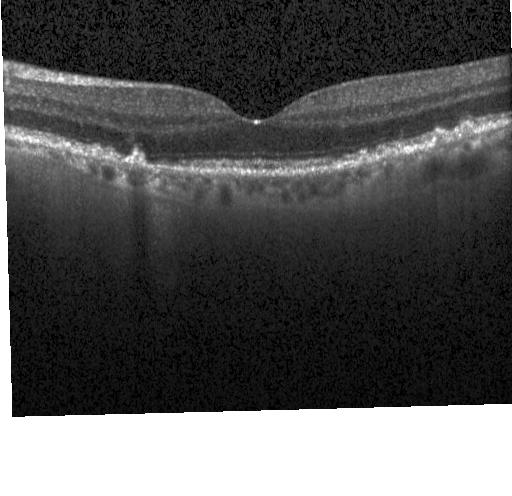
SD-OCT; centered on the fovea; OCT line scan; acquired on a Heidelberg Spectralis — Macular OCT: multiple drusen.